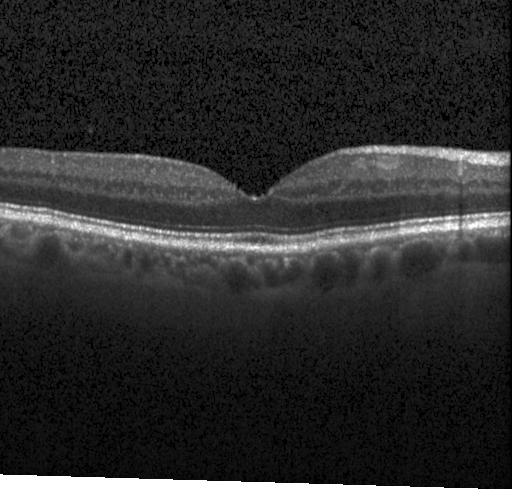

Instrument: Heidelberg Spectralis; spectral-domain optical coherence tomography; OCT line scan; horizontal scan through the fovea. Finding: no evidence of CNV, DME, or drusen.